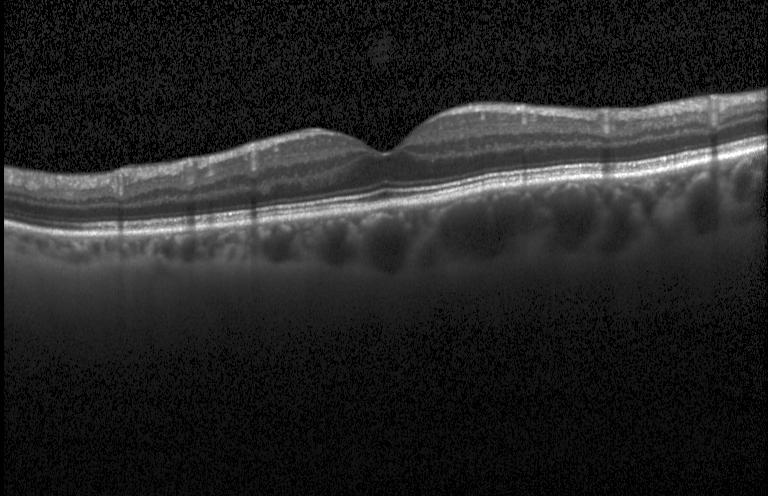

Retinal OCT cross-section showing no evidence of choroidal neovascularization, diabetic macular edema, or drusen.